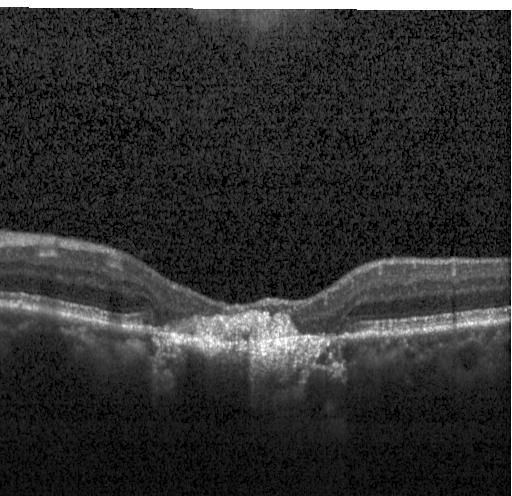 OCT line scan.
Finding: choroidal neovascularization.